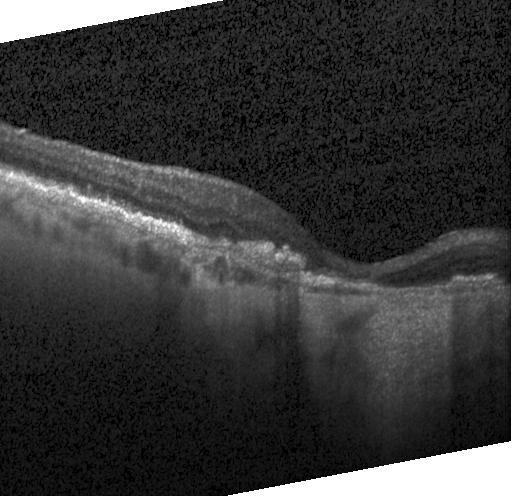
Centered on the fovea; retinal OCT cross-section
Dx: choroidal neovascularization.